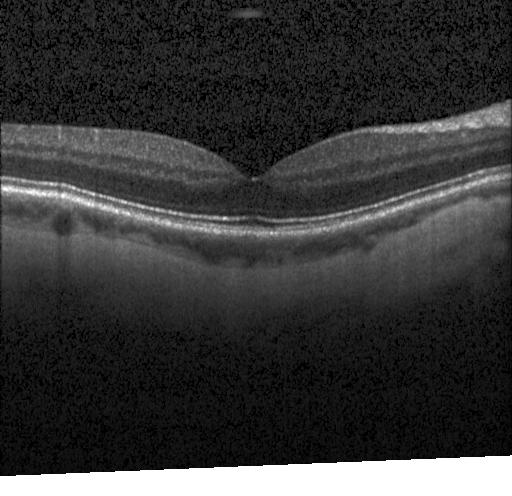 OCT B-scan · centered on the fovea — Dx: no CNV, DME, or drusen.